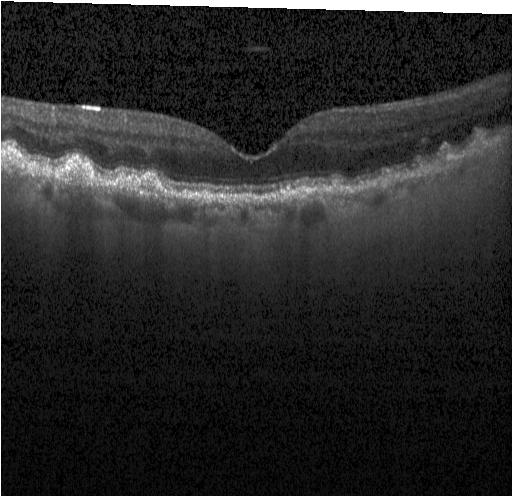

Retinal OCT B-scan; spectral-domain OCT; through the macula
The scan shows multiple drusen.